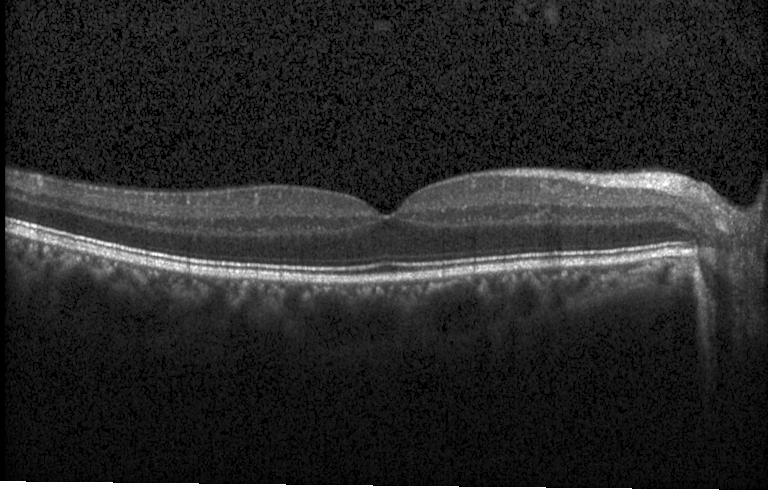

Finding: no evidence of choroidal neovascularization, diabetic macular edema, or drusen.